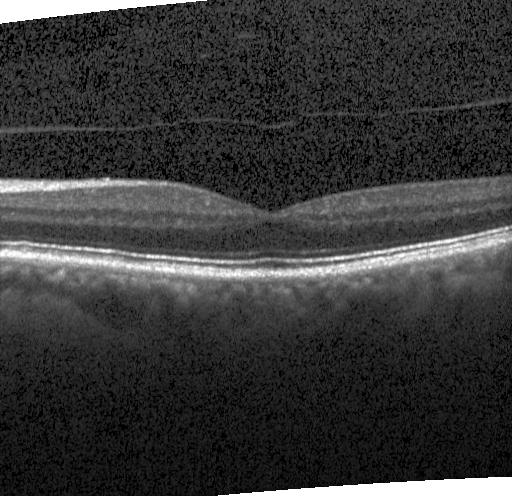
OCT B-scan showing no choroidal neovascularization, diabetic macular edema, or drusen.